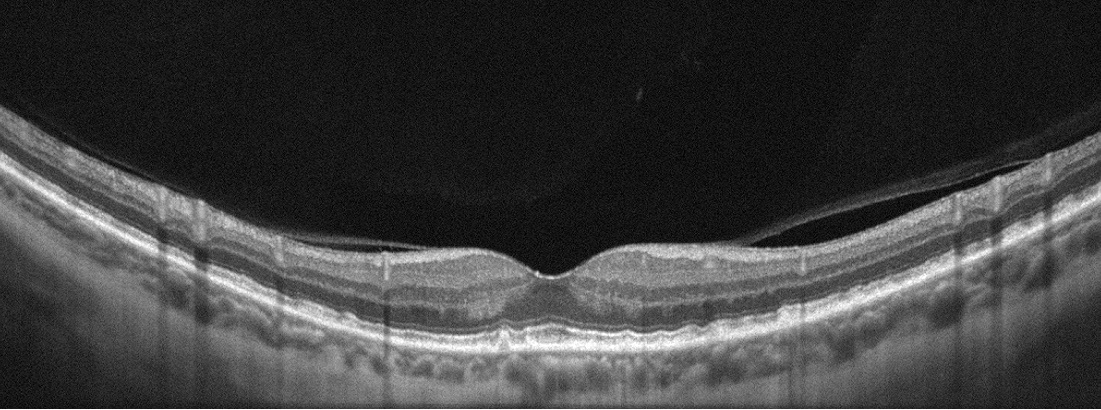
Acquired on an Optovue Avanti RTVue XR · optical coherence tomography scan
Diagnosis: age-related macular degeneration (AMD).